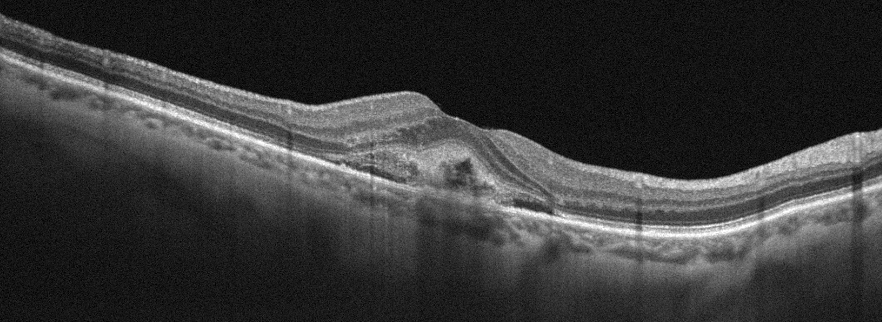 Macular scan; OCT B-scan; left eye — This B-scan demonstrates age-related macular degeneration.